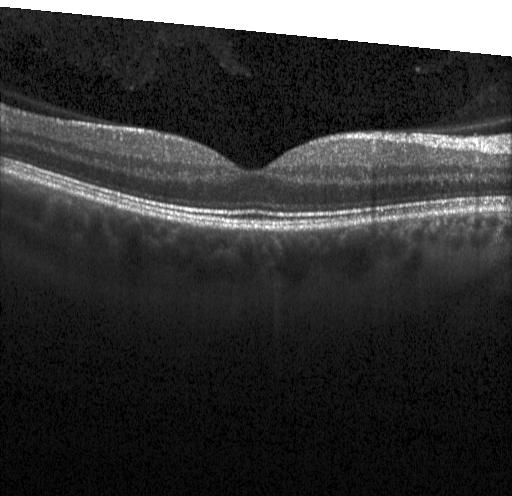
Centered on the fovea, optical coherence tomography B-scan, spectral-domain optical coherence tomography.
Macular OCT: no choroidal neovascularization, diabetic macular edema, or drusen.